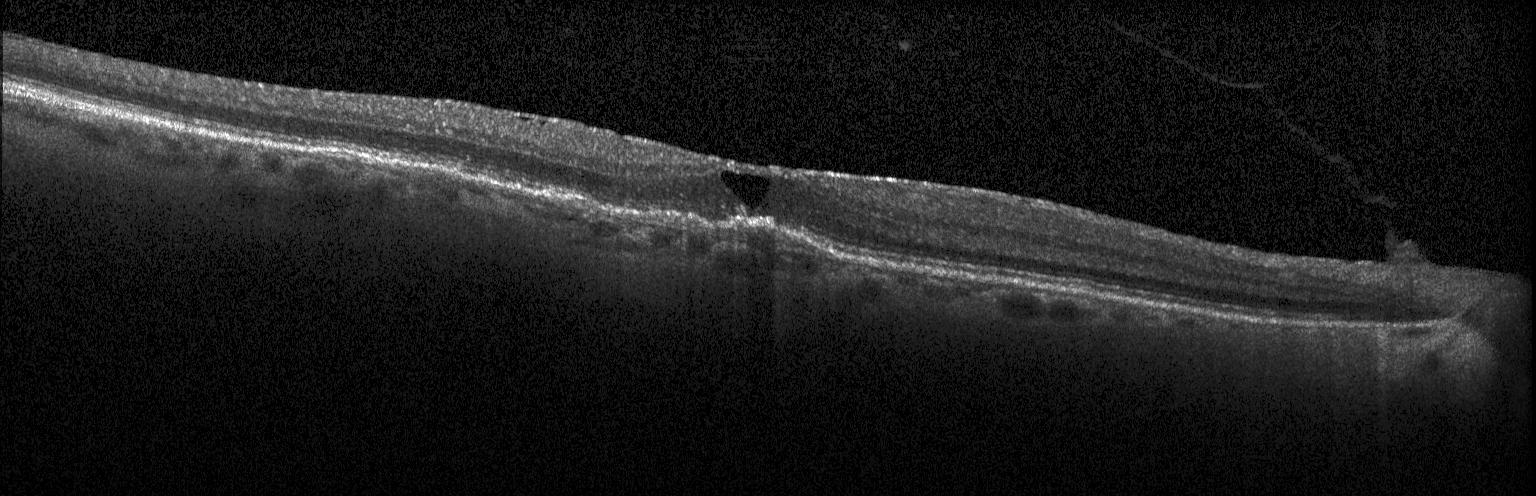

Retinal OCT B-scan; horizontal scan through the fovea.
Assessment: choroidal neovascularization (CNV).